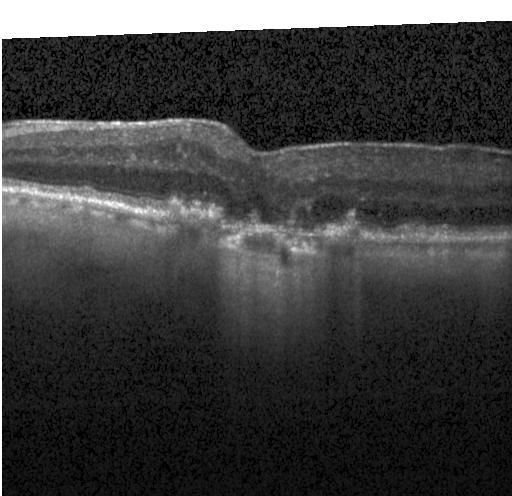
Macular scan · optical coherence tomography scan
Diagnosis: a choroidal neovascular membrane.